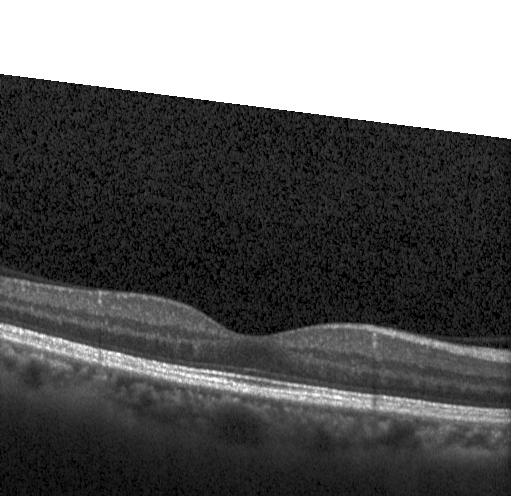

Assessment: no evidence of CNV, DME, or drusen.